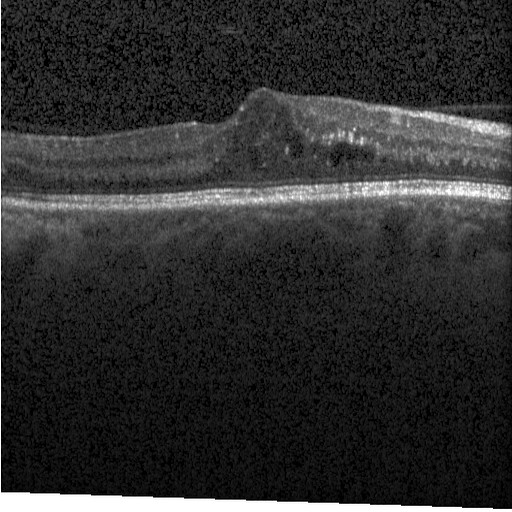
OCT B-scan; acquired on a Heidelberg Spectralis; horizontal scan through the fovea
Diagnosis: diabetic macular edema (DME).